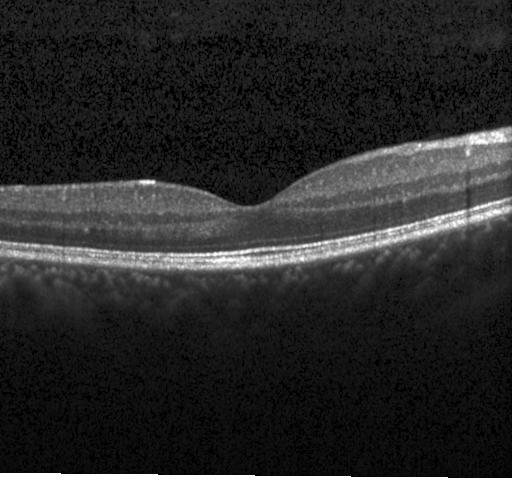

Spectral-domain optical coherence tomography. Optical coherence tomography scan — Impression: no choroidal neovascularization, no diabetic macular edema, and no drusen.